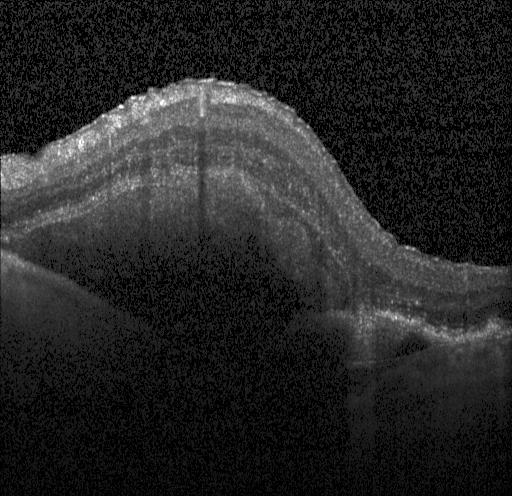
This B-scan demonstrates a choroidal neovascular membrane.